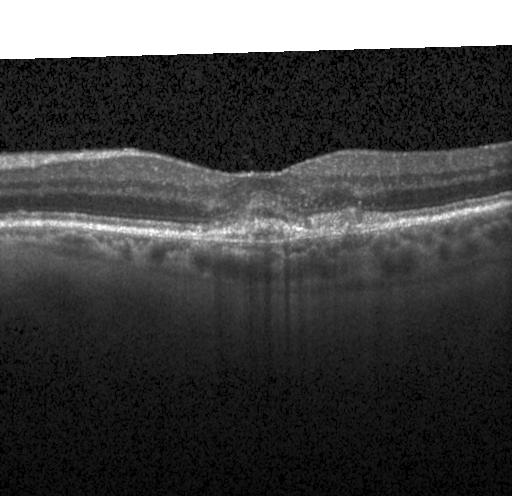
Macular scan · SD-OCT · OCT B-scan · instrument: Heidelberg Spectralis.
Diagnosis: choroidal neovascularization (CNV).